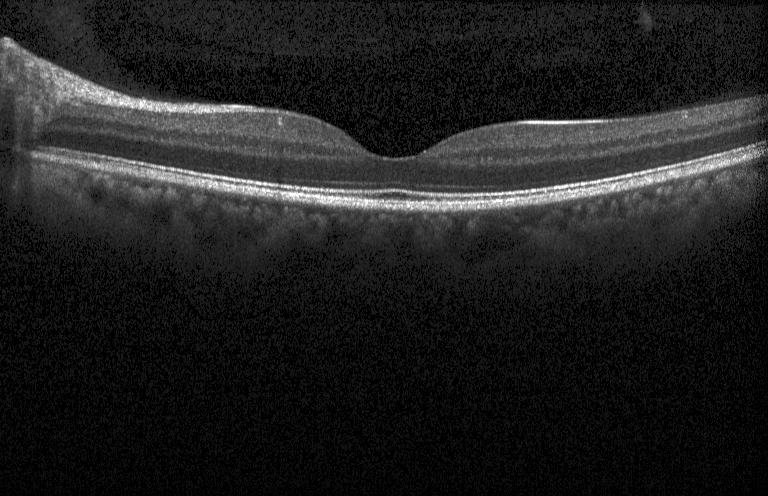 Heidelberg Spectralis. Optical coherence tomography B-scan.
The scan shows neither CNV, DME, nor drusen.